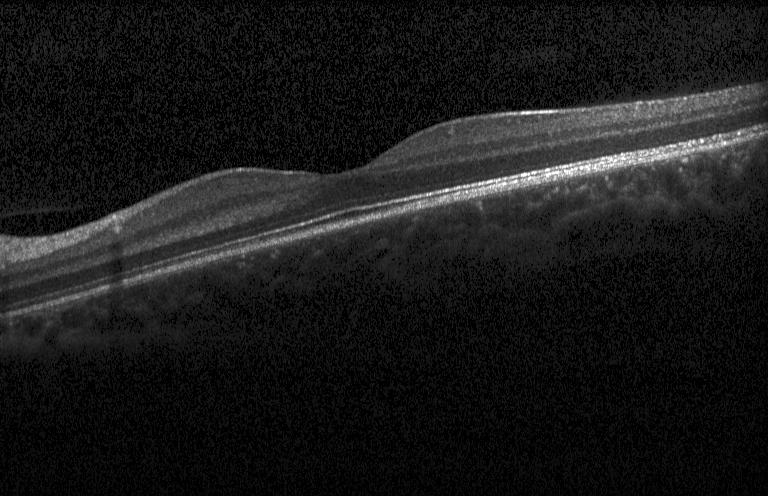 OCT line scan · spectral-domain optical coherence tomography · acquired on a Heidelberg Spectralis. Diagnosis: no CNV, DME, or drusen.